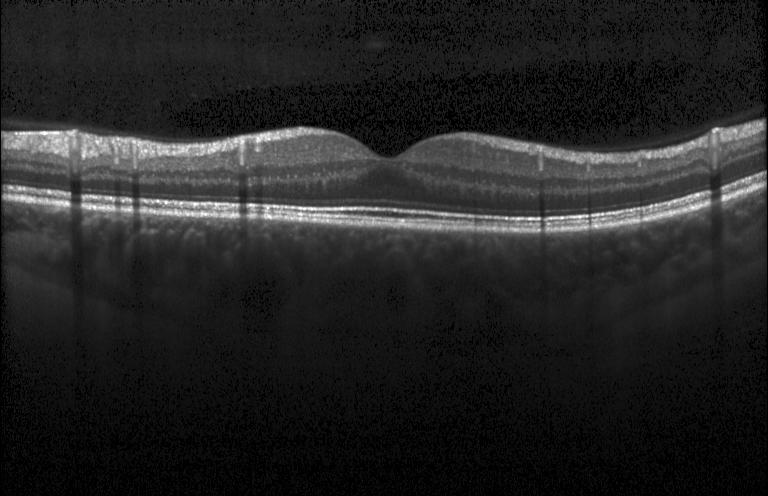 Retinal OCT B-scan.
Neither CNV, DME, nor drusen.